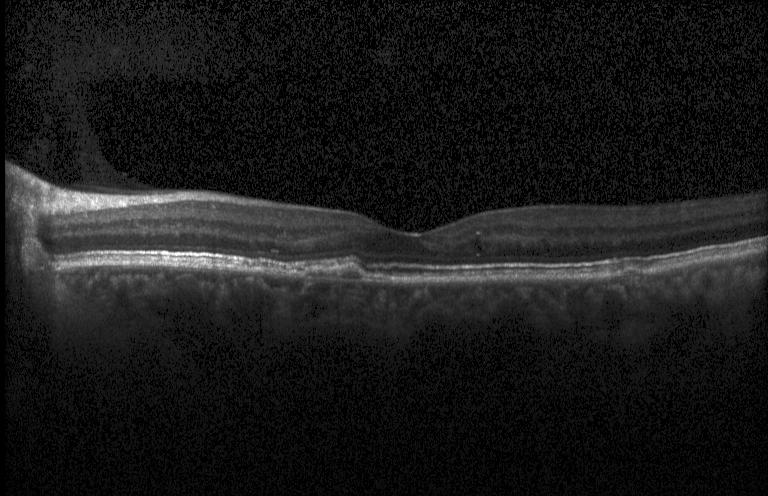

OCT B-scan, acquired on a Heidelberg Spectralis — This B-scan demonstrates CNV.